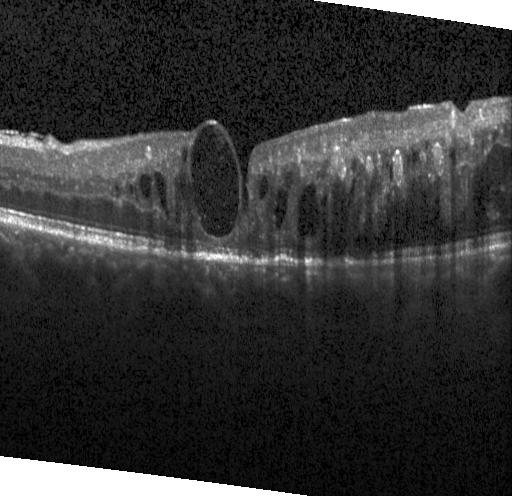 Finding: diabetic macular edema.